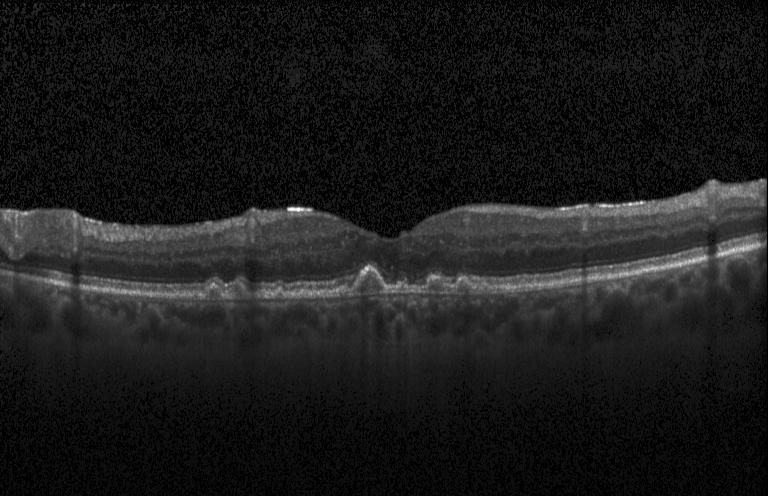

Retinal OCT cross-section; macular scan; instrument: Heidelberg Spectralis. Finding: drusen.